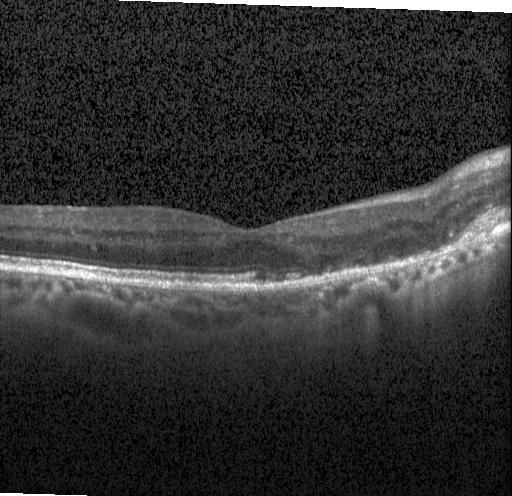
Optical coherence tomography B-scan; instrument: Heidelberg Spectralis; spectral-domain OCT. Impression: a choroidal neovascular membrane.